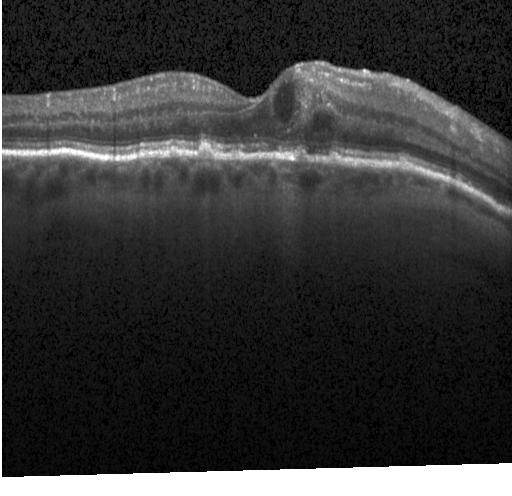
Assessment: CNV.